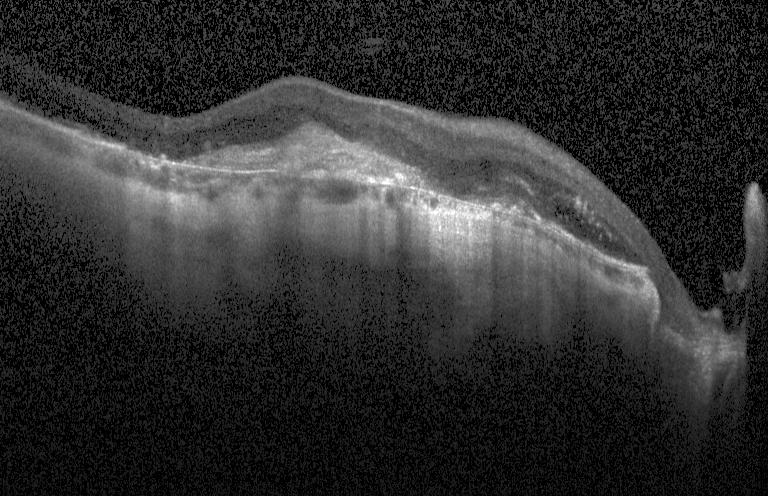 Spectral-domain optical coherence tomography, retinal OCT cross-section, instrument: Heidelberg Spectralis
Impression: a choroidal neovascular membrane.